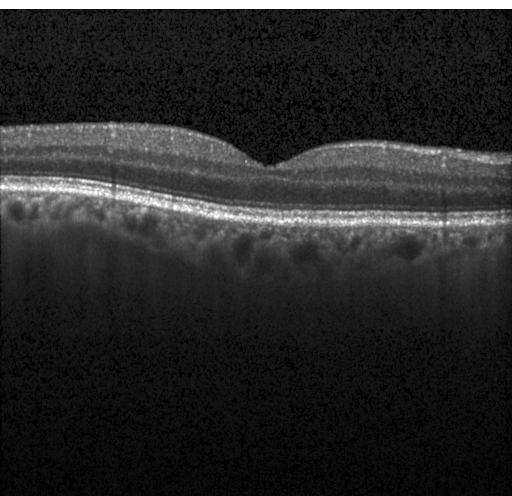

Impression: no choroidal neovascularization, diabetic macular edema, or drusen.